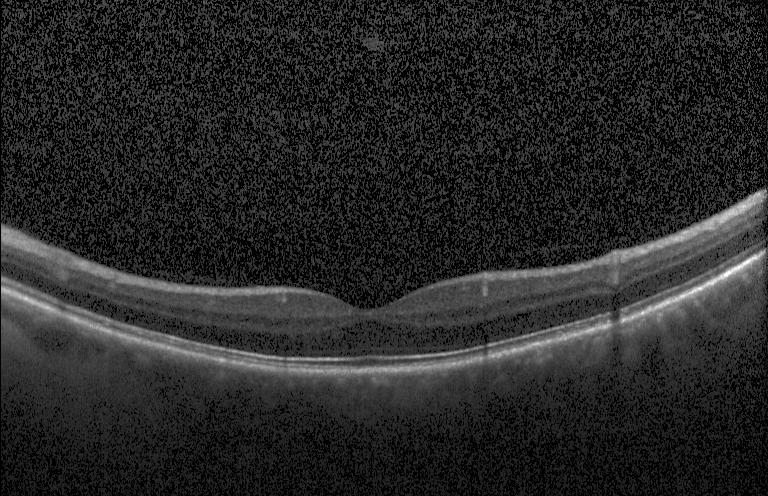
OCT B-scan.
Diagnosis: no choroidal neovascularization, no diabetic macular edema, and no drusen.